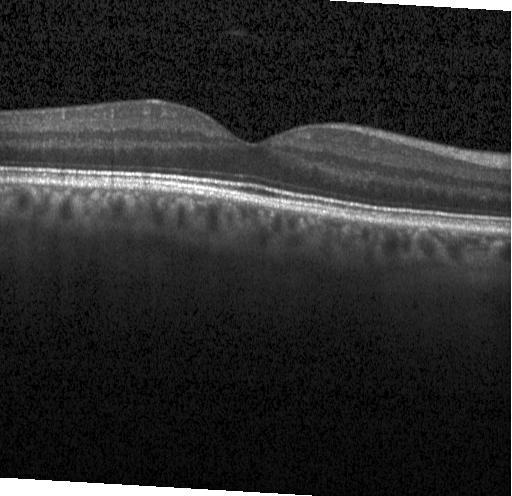

Retinal OCT B-scan; Heidelberg Spectralis OCT system
Diagnosis: no CNV, no DME, and no drusen.